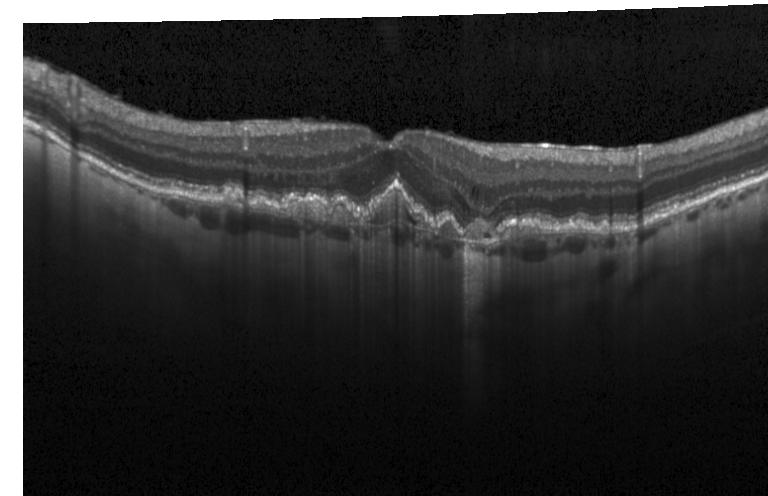
SD-OCT; optical coherence tomography B-scan — Assessment: a choroidal neovascular membrane.